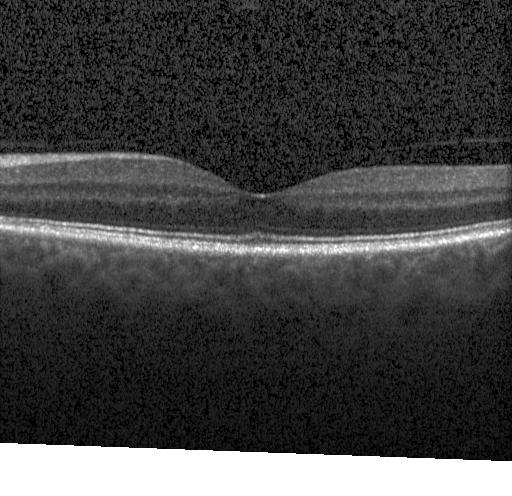 Optical coherence tomography scan; acquired on a Heidelberg Spectralis.
OCT finding: no evidence of choroidal neovascularization, diabetic macular edema, or drusen.